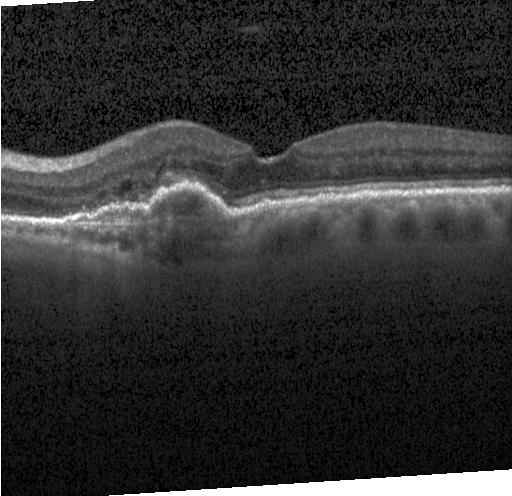 Optical coherence tomography B-scan — This B-scan demonstrates a choroidal neovascular membrane.